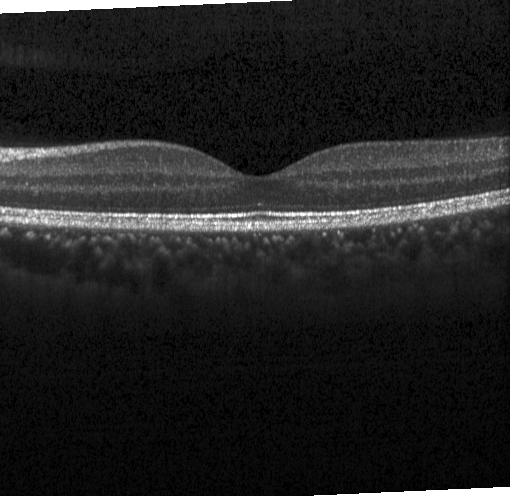

Optical coherence tomography B-scan — This B-scan demonstrates no evidence of choroidal neovascularization, diabetic macular edema, or drusen.